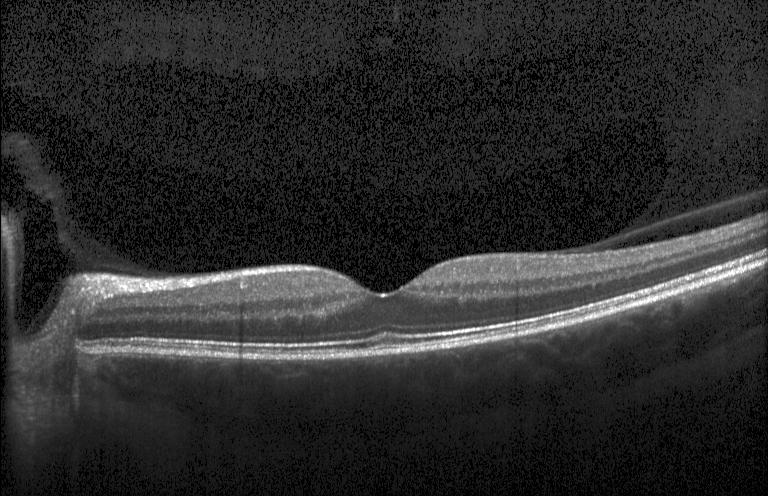
OCT B-scan showing no choroidal neovascularization, no diabetic macular edema, and no drusen.